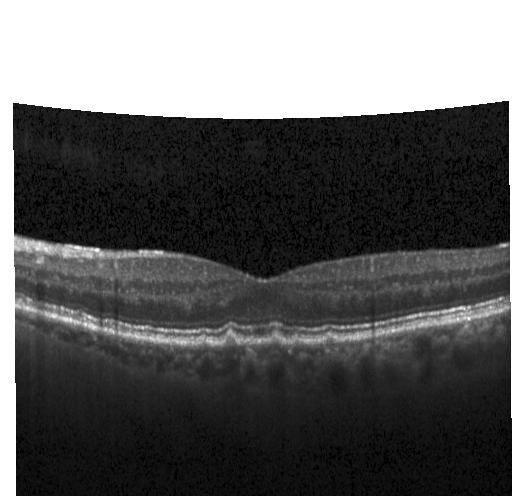 Impression: multiple drusen.